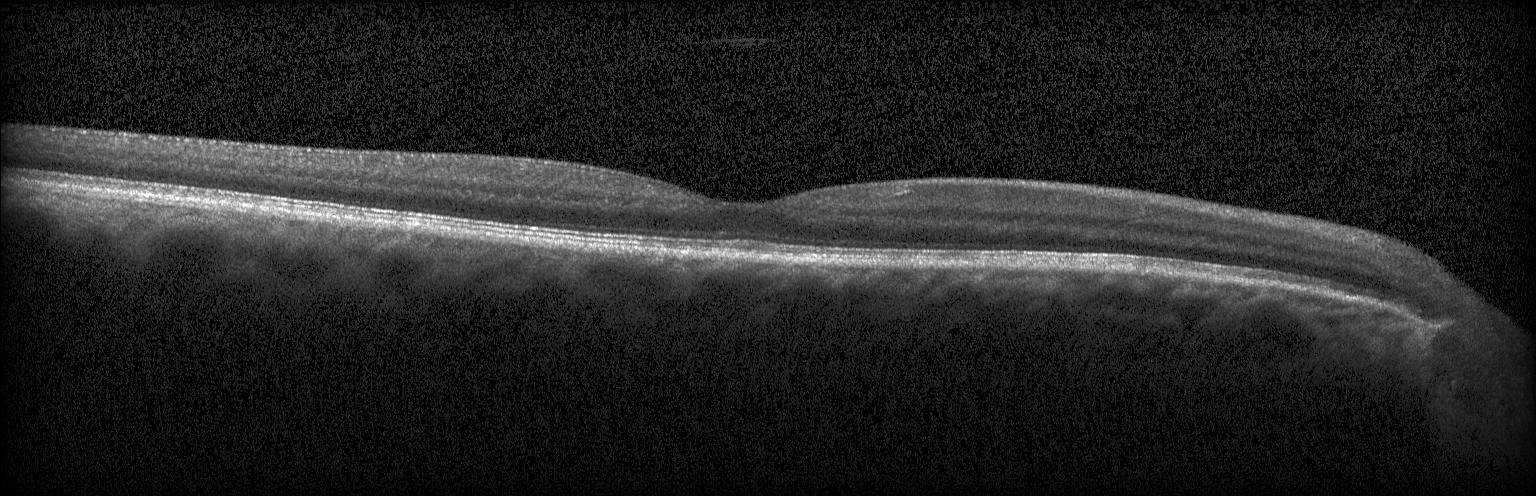

This B-scan demonstrates no evidence of CNV, DME, or drusen.